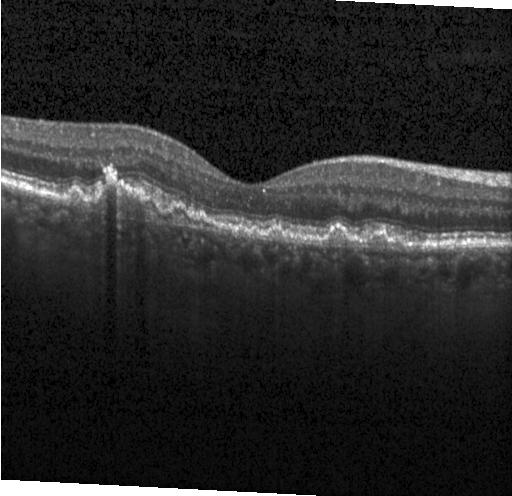

Assessment: choroidal neovascularization.